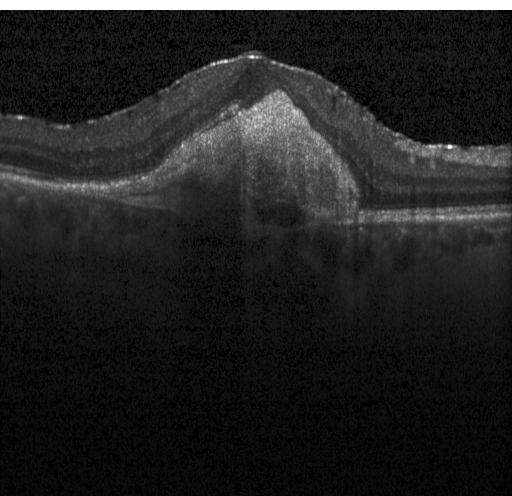
Macular scan. Instrument: Heidelberg Spectralis. Spectral-domain optical coherence tomography. OCT B-scan. Diagnosis: a choroidal neovascular membrane.